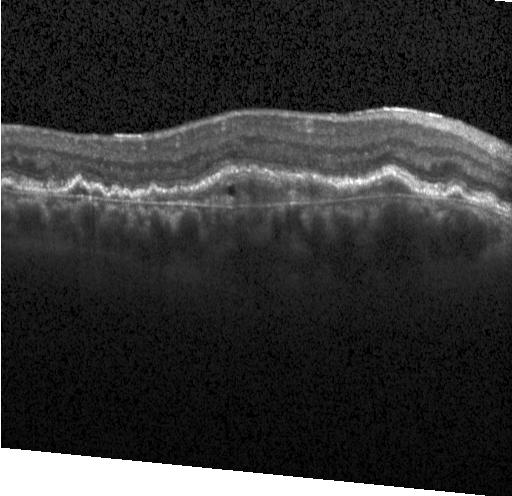
Retinal OCT B-scan
This B-scan demonstrates choroidal neovascularization.